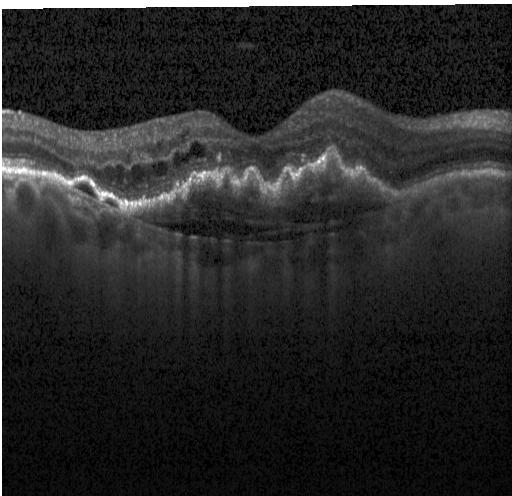
Acquired on a Heidelberg Spectralis · macular scan · SD-OCT · retinal OCT B-scan — The scan shows CNV.